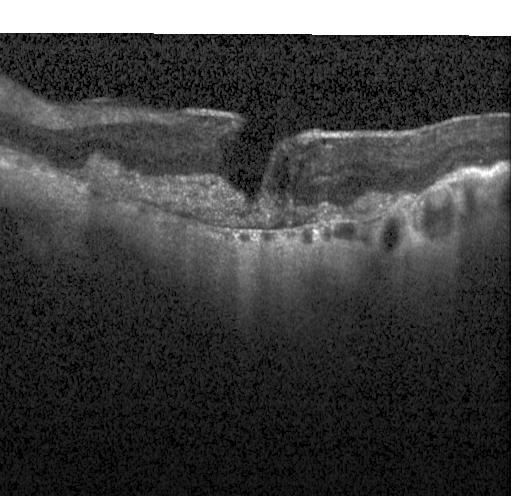 Macular OCT demonstrating CNV.